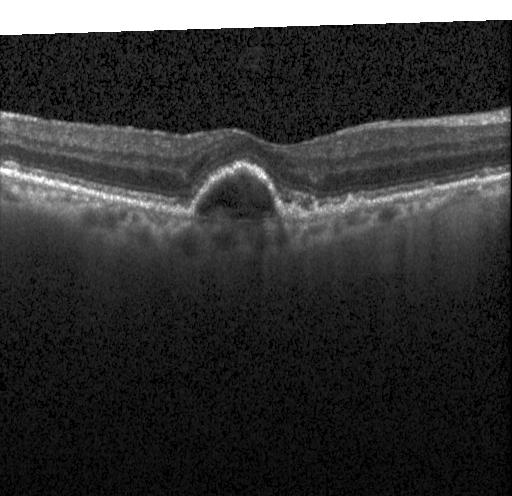
Through the macula, OCT B-scan, spectral-domain OCT — This B-scan demonstrates CNV.